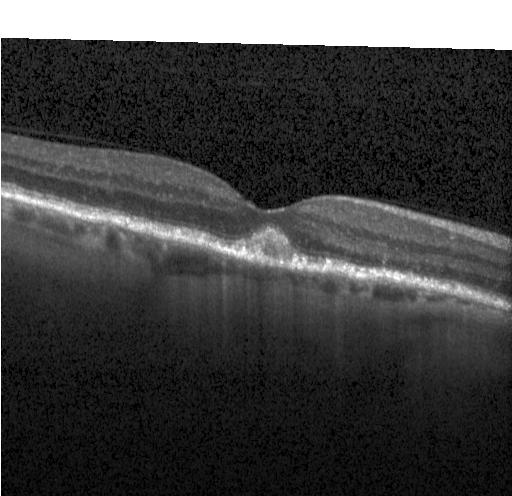 Retinal OCT B-scan. Diagnosis: drusen.